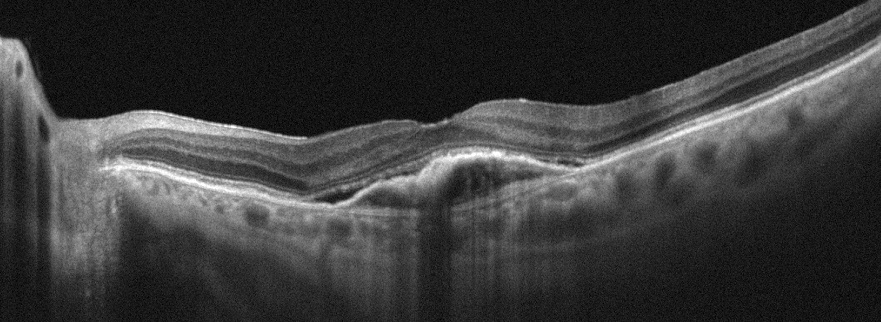

Impression: AMD.